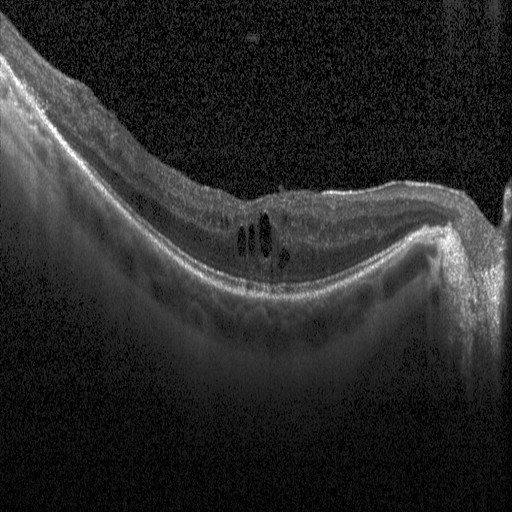
Diabetic macular edema.